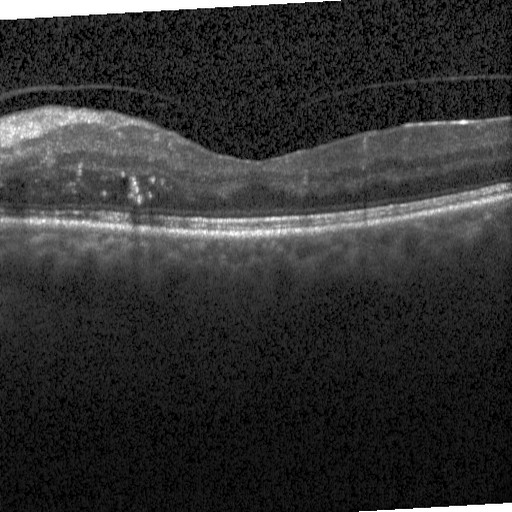
OCT B-scan; spectral-domain optical coherence tomography; horizontal scan through the fovea; Heidelberg Spectralis — Diagnosis: DME.